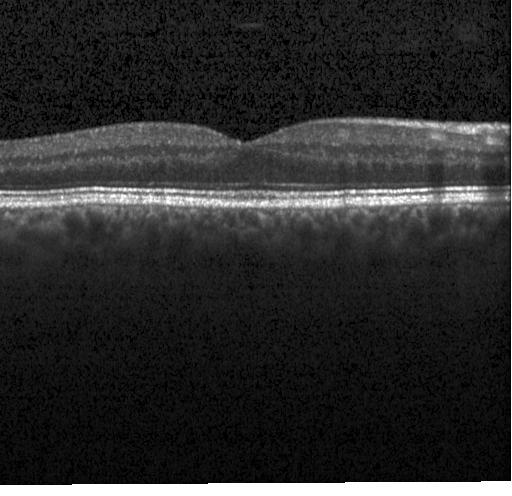 OCT B-scan · spectral-domain optical coherence tomography · centered on the fovea.
This B-scan demonstrates no choroidal neovascularization, diabetic macular edema, or drusen.